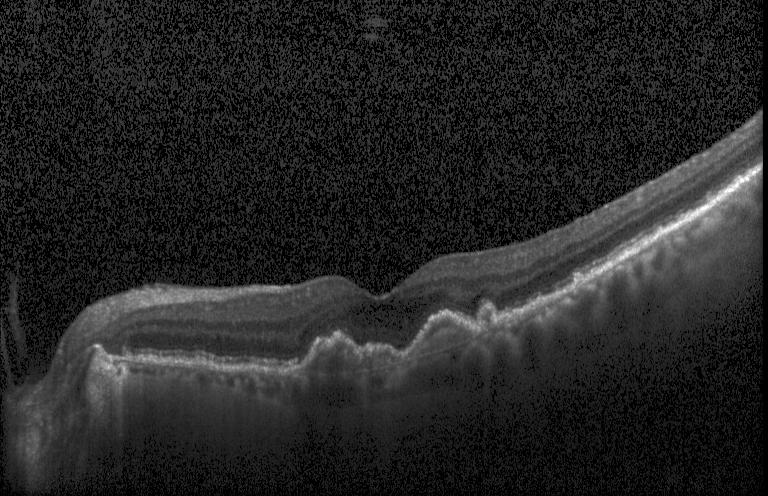 Heidelberg Spectralis; optical coherence tomography B-scan — Dx: a choroidal neovascular membrane.